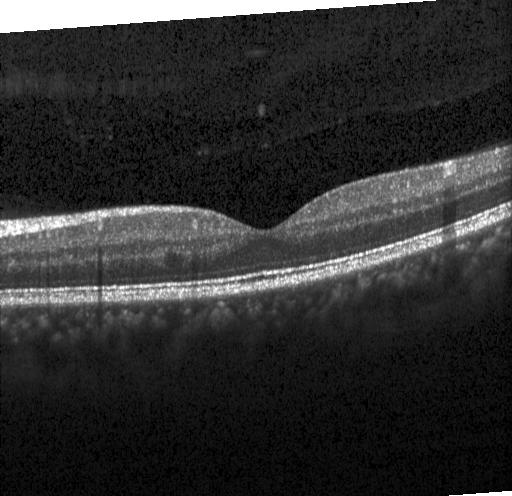

OCT B-scan showing neither CNV, DME, nor drusen.